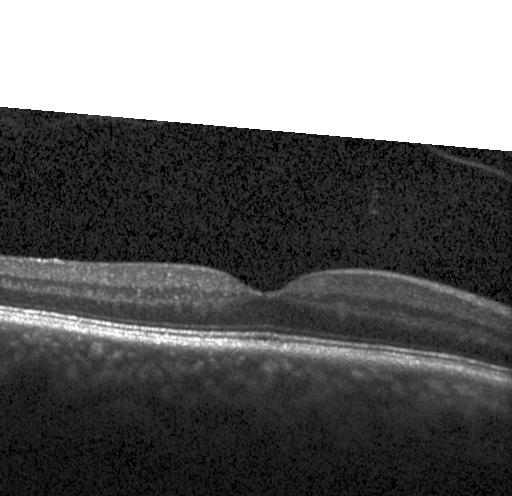 Through the macula. OCT B-scan. Spectral-domain optical coherence tomography. Instrument: Heidelberg Spectralis. Impression: no CNV, DME, or drusen.